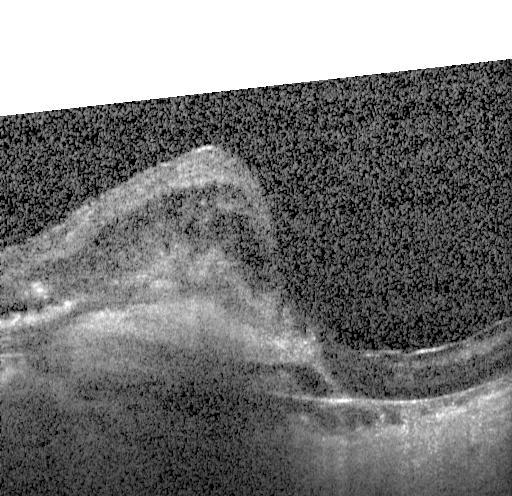

OCT line scan, SD-OCT
Diagnosis: choroidal neovascularization.